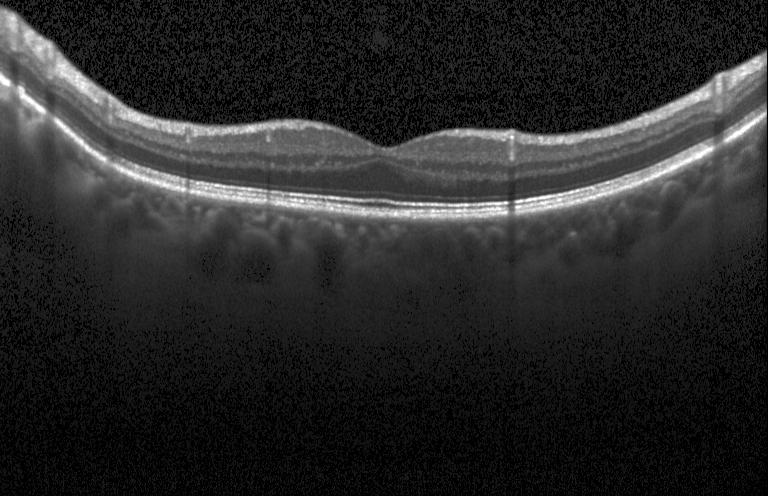 Horizontal scan through the fovea, spectral-domain OCT, optical coherence tomography scan, Heidelberg Spectralis OCT system
Neither choroidal neovascularization, diabetic macular edema, nor drusen.